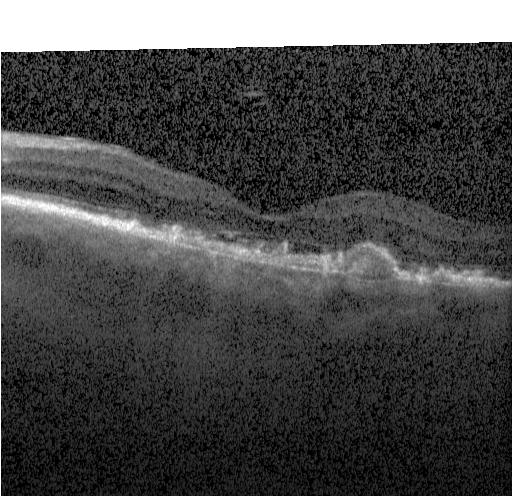
The scan shows choroidal neovascularization (CNV).